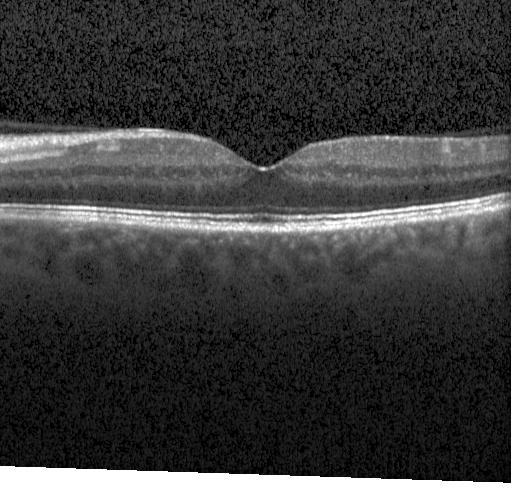 Acquired on a Heidelberg Spectralis; OCT B-scan; fovea-centered.
This B-scan demonstrates no CNV, DME, or drusen.